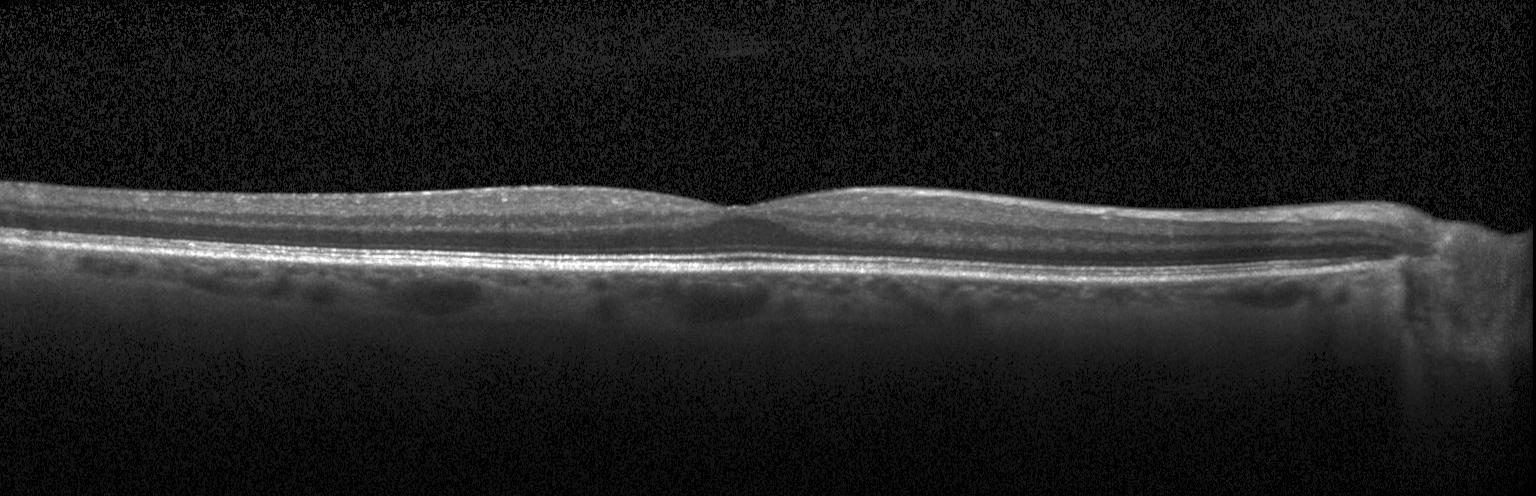 This B-scan demonstrates no choroidal neovascularization, diabetic macular edema, or drusen.